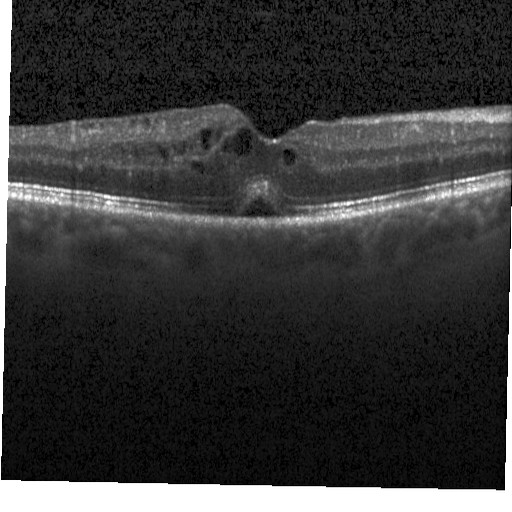

OCT B-scan, through the macula, spectral-domain OCT. Diagnosis: diabetic macular edema.